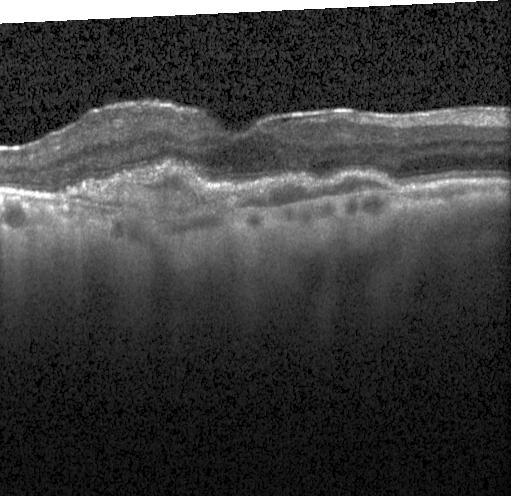
OCT line scan.
Impression: a choroidal neovascular membrane.